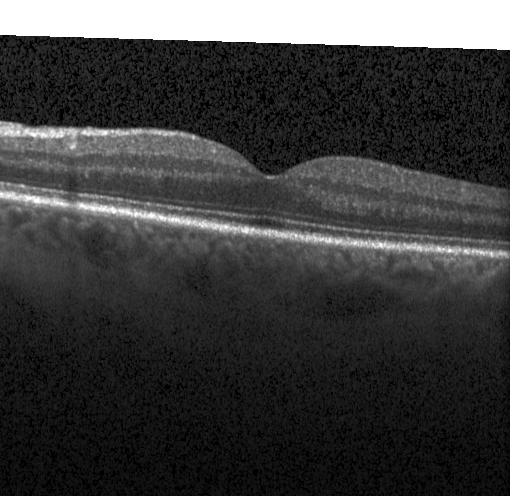

Heidelberg Spectralis. Horizontal scan through the fovea. Optical coherence tomography B-scan. Spectral-domain OCT. Diagnosis: neither CNV, DME, nor drusen.